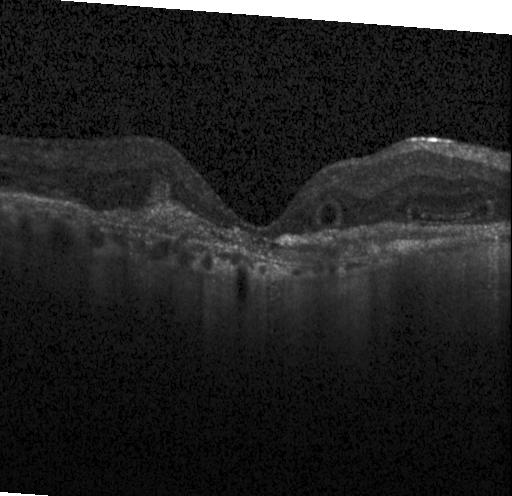
A choroidal neovascular membrane.